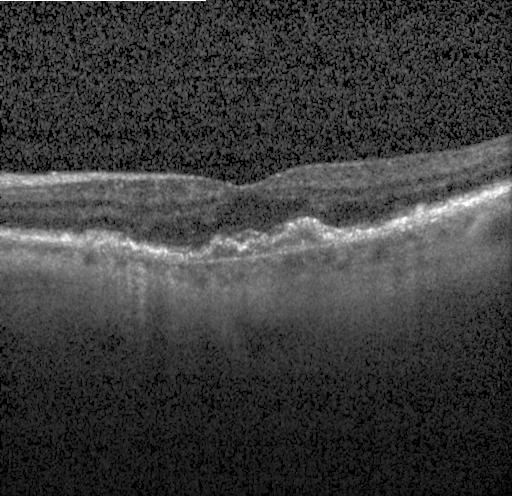
Optical coherence tomography B-scan
Finding: a choroidal neovascular membrane.